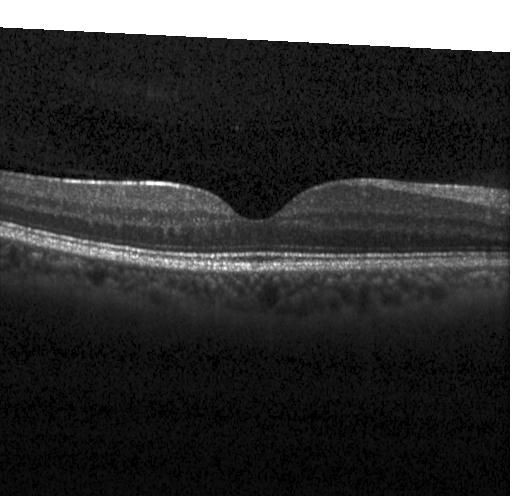 Retinal OCT B-scan; spectral-domain optical coherence tomography; instrument: Heidelberg Spectralis.
Impression: neither choroidal neovascularization, diabetic macular edema, nor drusen.